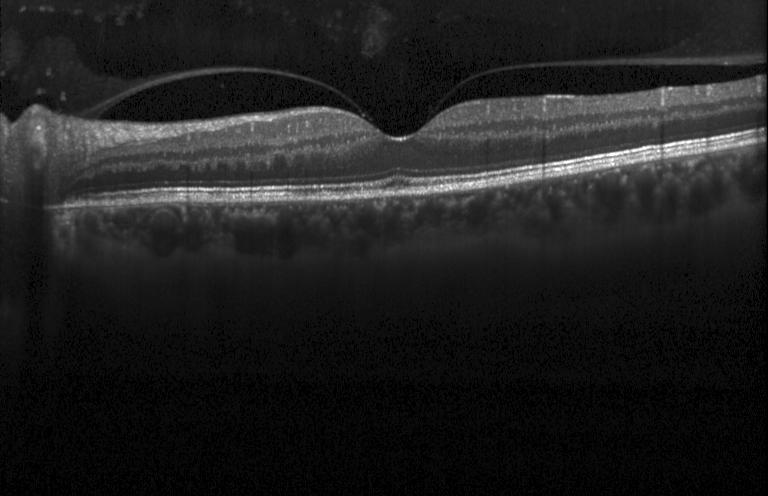 Through the macula. Optical coherence tomography scan.
The scan shows neither choroidal neovascularization, diabetic macular edema, nor drusen.